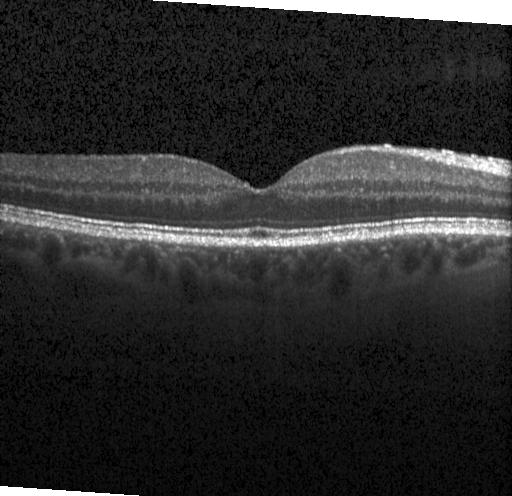
Spectral-domain OCT, Heidelberg Spectralis, optical coherence tomography scan — Dx: no choroidal neovascularization, diabetic macular edema, or drusen.